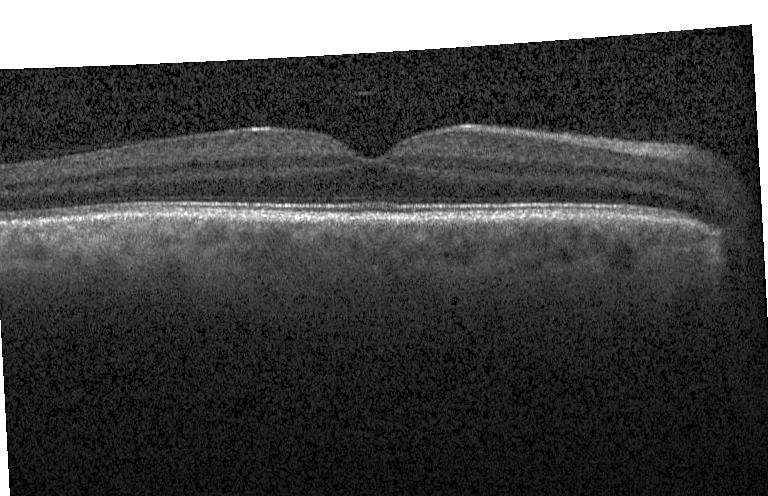 OCT B-scan showing no evidence of choroidal neovascularization, diabetic macular edema, or drusen.